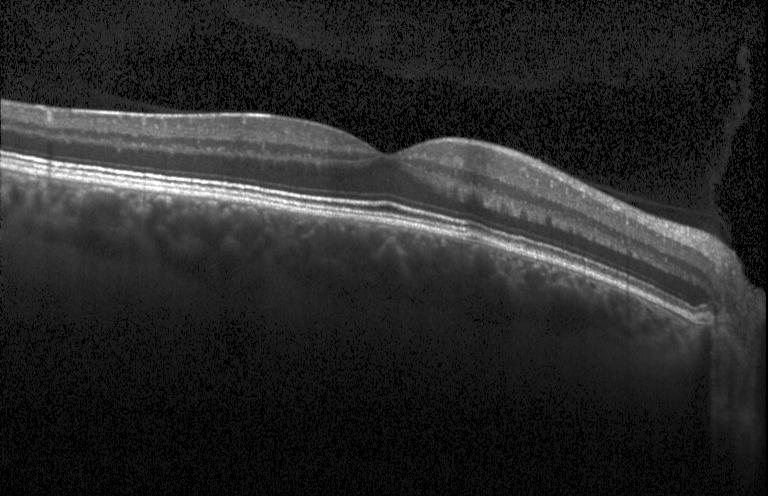

Spectral-domain OCT B-scan: no CNV, DME, or drusen.